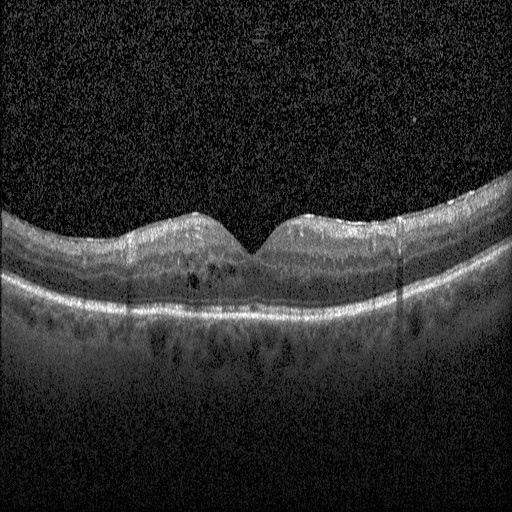 OCT B-scan showing diabetic macular edema.